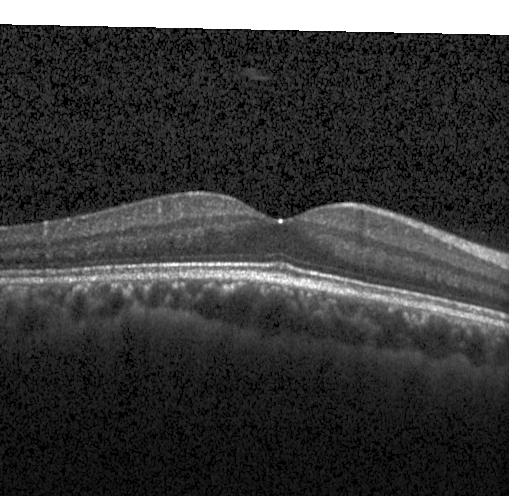
Optical coherence tomography scan — Diagnosis: neither choroidal neovascularization, diabetic macular edema, nor drusen.